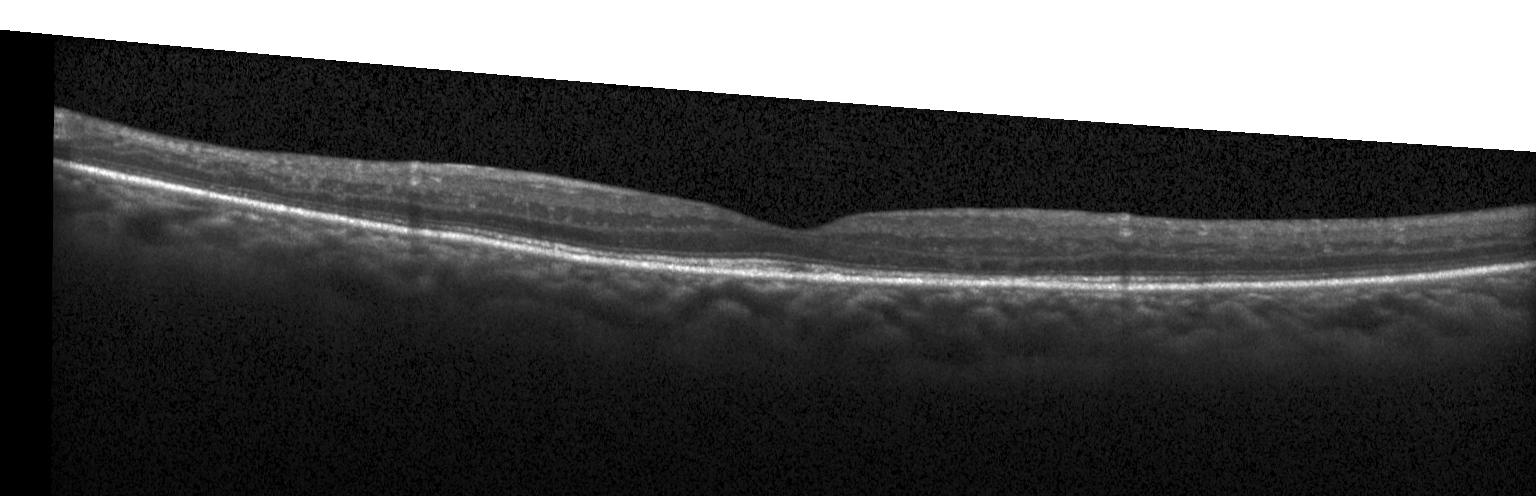

Instrument: Heidelberg Spectralis; spectral-domain OCT; optical coherence tomography B-scan.
This B-scan demonstrates no choroidal neovascularization, diabetic macular edema, or drusen.